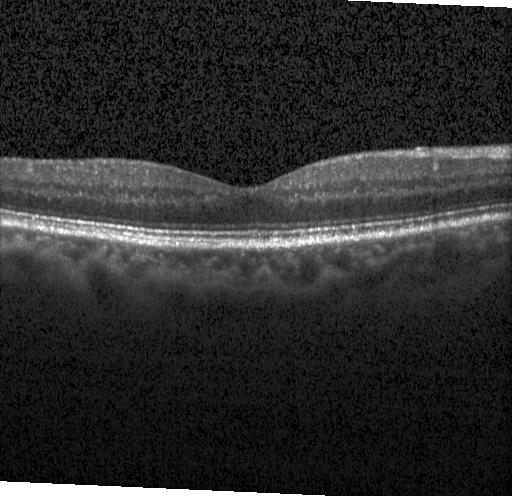 Optical coherence tomography scan. Heidelberg Spectralis. Spectral-domain OCT. Horizontal scan through the fovea.
Assessment: no choroidal neovascularization, no diabetic macular edema, and no drusen.